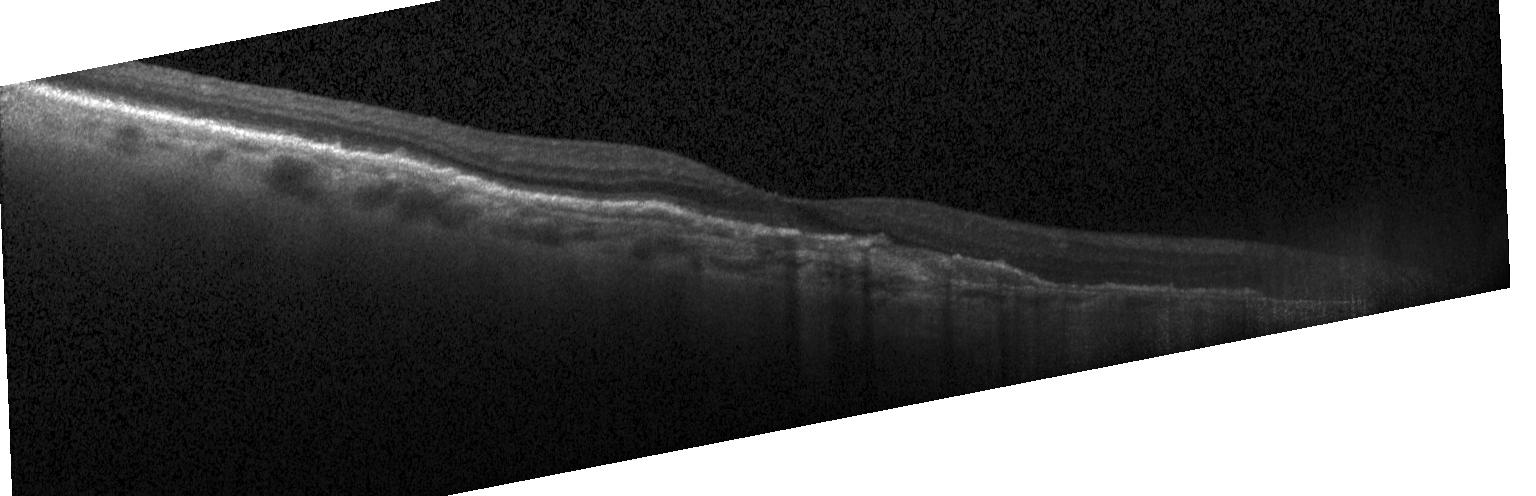
Spectral-domain OCT; optical coherence tomography B-scan; horizontal scan through the fovea.
Macular OCT: a choroidal neovascular membrane.